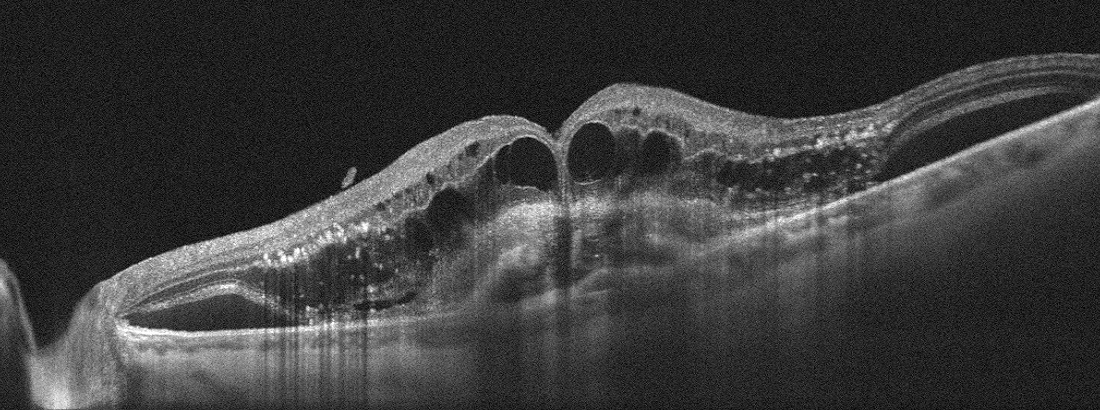 The scan shows age-related macular degeneration.